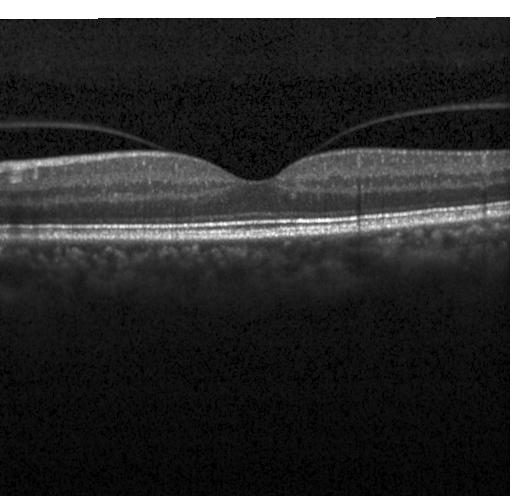
The scan shows no CNV, no DME, and no drusen.